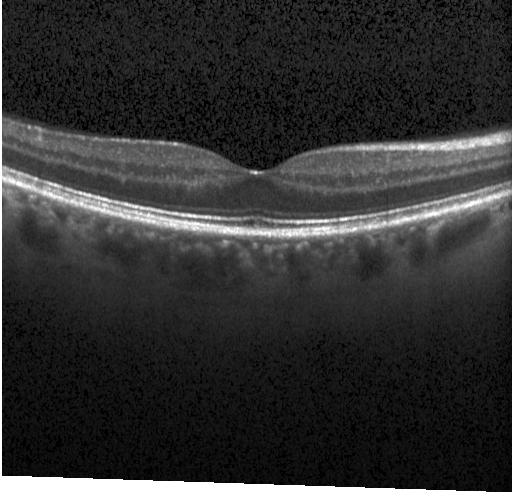

OCT finding: no CNV, no DME, and no drusen.